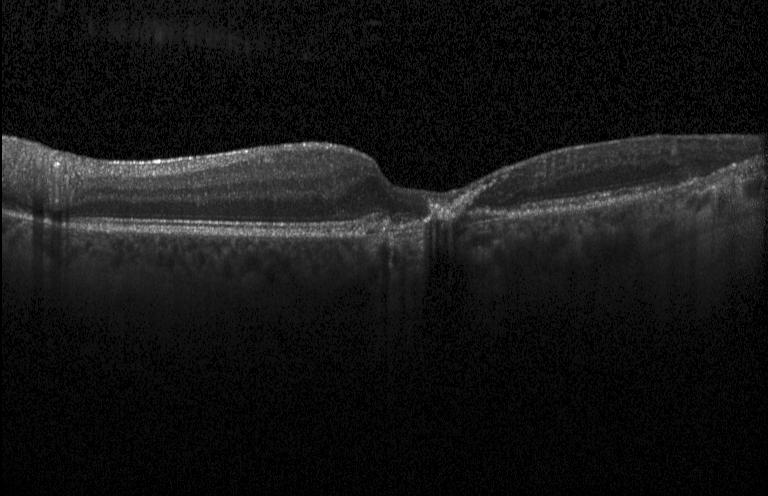
OCT line scan — Impression: choroidal neovascularization (CNV).